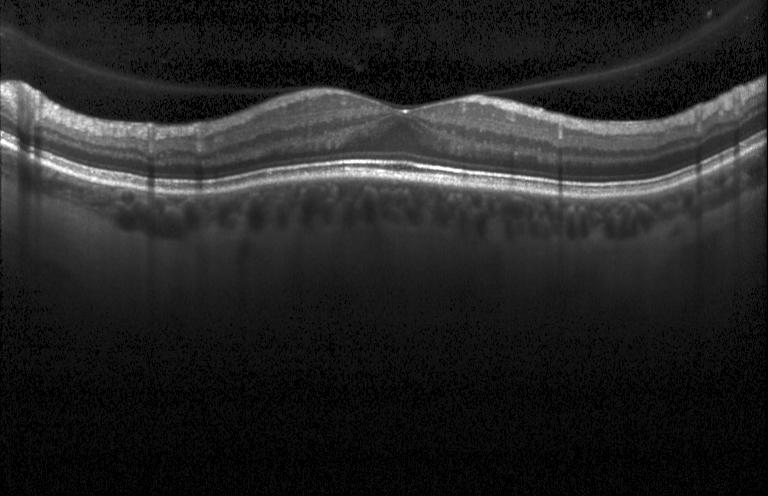

Assessment: no CNV, no DME, and no drusen.